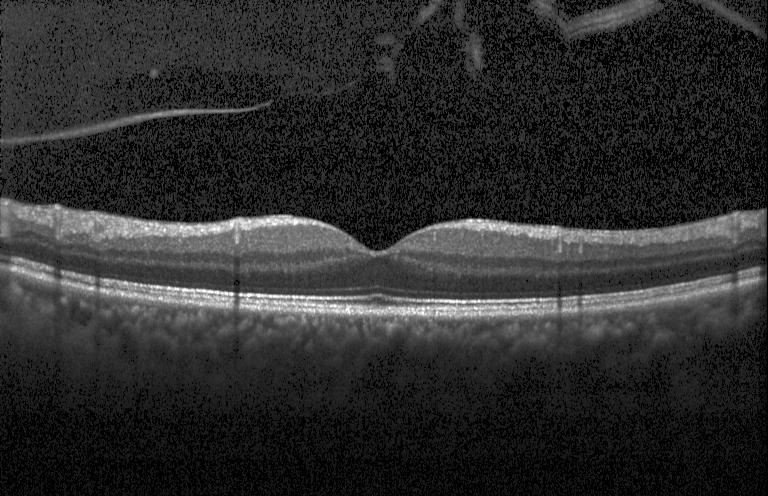
Impression: no evidence of choroidal neovascularization, diabetic macular edema, or drusen.